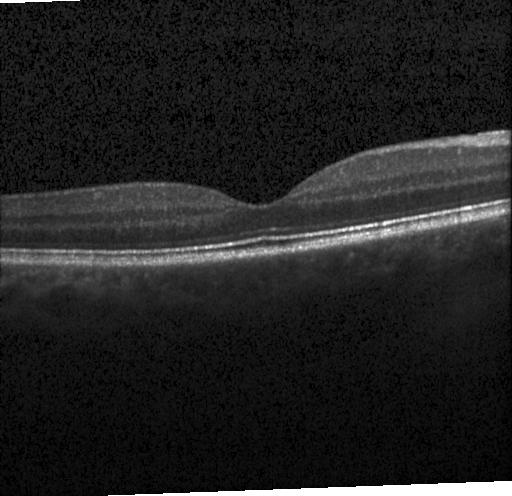

Spectral-domain OCT, fovea-centered, Heidelberg Spectralis OCT system, retinal OCT B-scan — Dx: neither choroidal neovascularization, diabetic macular edema, nor drusen.